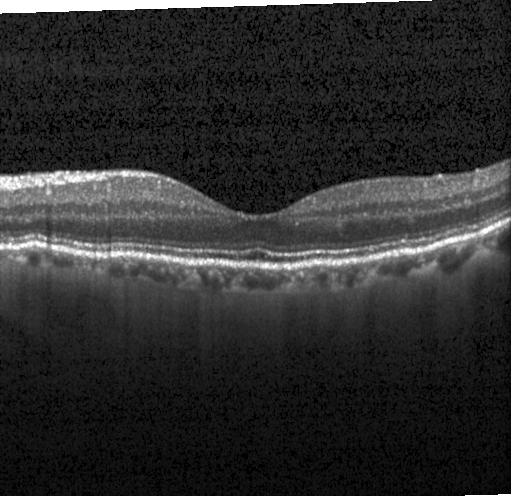
Acquired on a Heidelberg Spectralis; through the macula; optical coherence tomography B-scan
Diagnosis: neither choroidal neovascularization, diabetic macular edema, nor drusen.